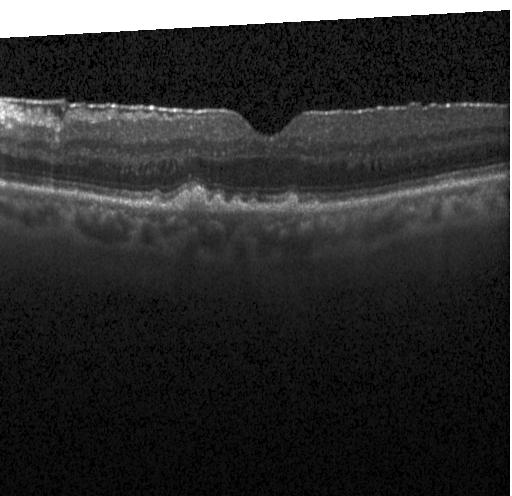

This B-scan demonstrates drusen.